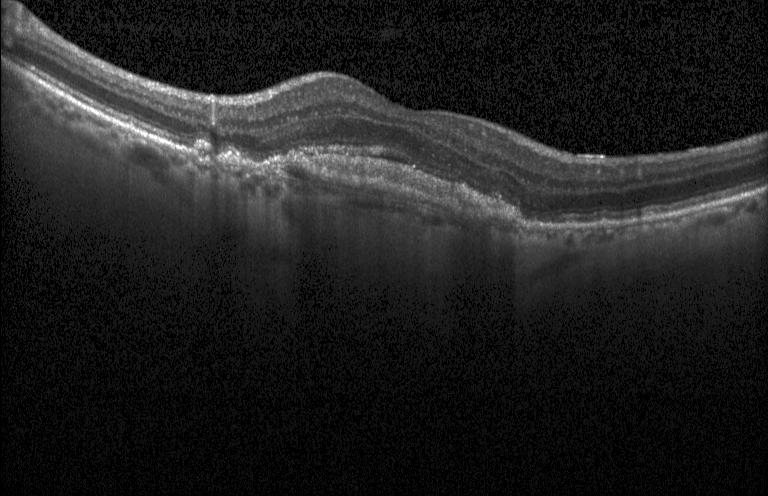 Optical coherence tomography B-scan
This B-scan demonstrates a choroidal neovascular membrane.